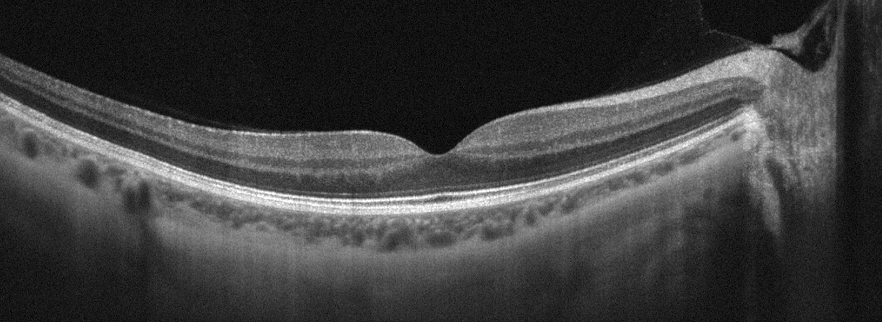 Oculus dexter. Optical coherence tomography B-scan. Impression: no AMD, DME, ERM, RAO, RVO, or VID.